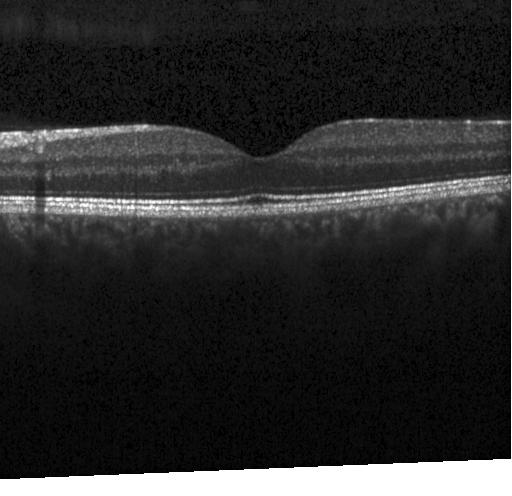

Retinal OCT cross-section · fovea-centered.
Finding: no CNV, no DME, and no drusen.